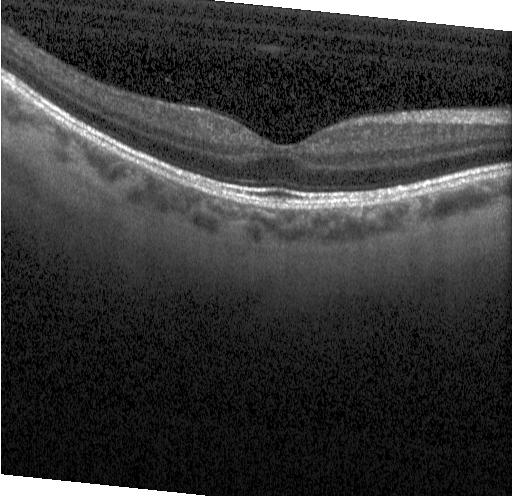
OCT B-scan
Impression: no choroidal neovascularization, diabetic macular edema, or drusen.